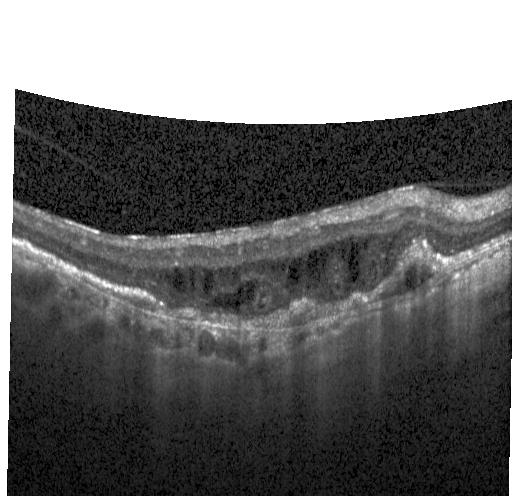
Centered on the fovea · spectral-domain OCT · OCT line scan. Diagnosis: choroidal neovascularization.